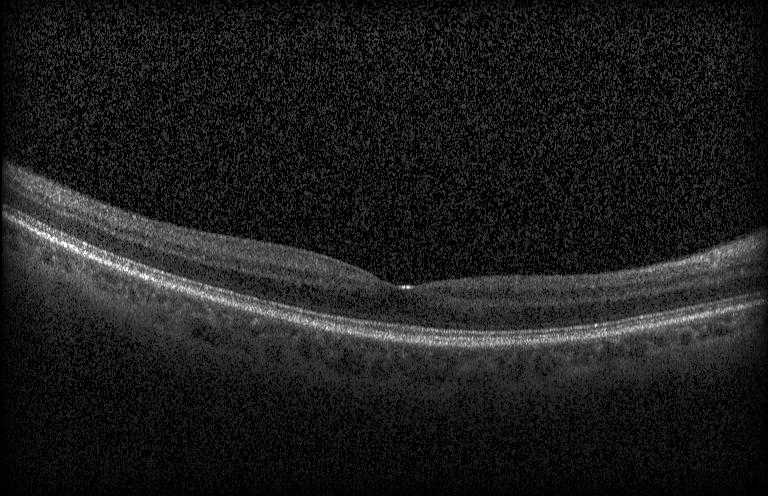

Impression: no CNV, DME, or drusen.